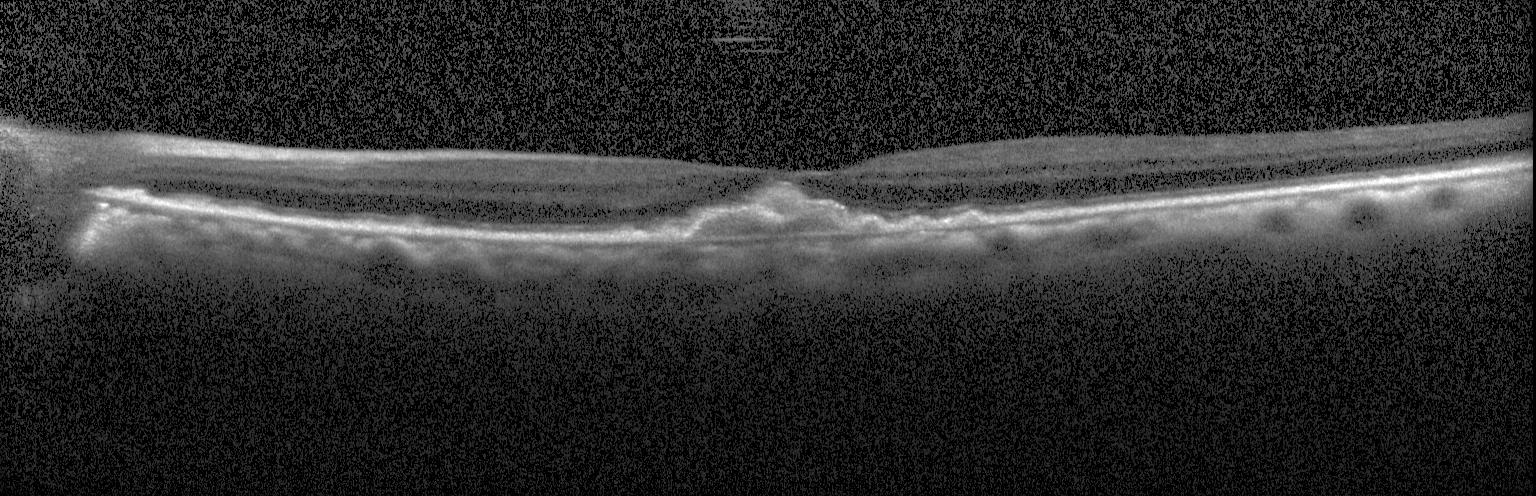
OCT scan showing a choroidal neovascular membrane.